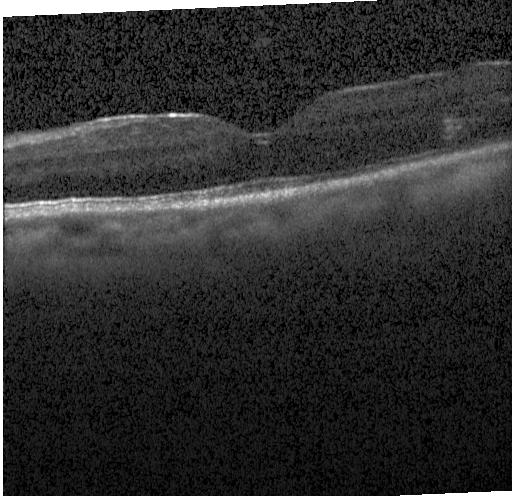
Heidelberg Spectralis OCT system; retinal OCT B-scan; spectral-domain OCT.
Dx: no CNV, DME, or drusen.